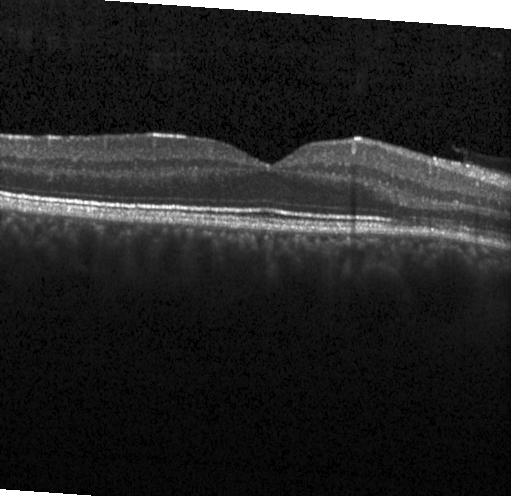 Horizontal scan through the fovea. Heidelberg Spectralis OCT system. Spectral-domain OCT. Retinal OCT cross-section
Diagnosis: no CNV, DME, or drusen.